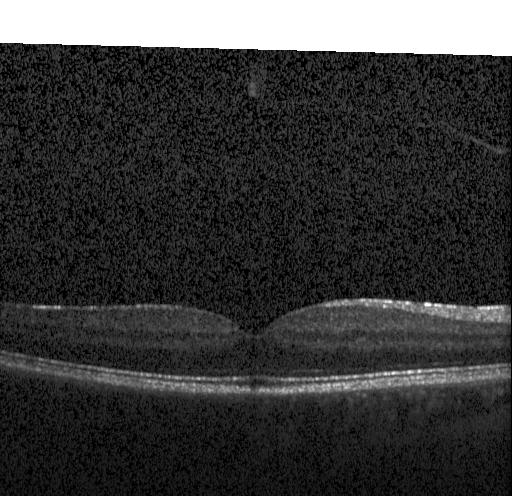
Retinal OCT cross-section showing no choroidal neovascularization, diabetic macular edema, or drusen.